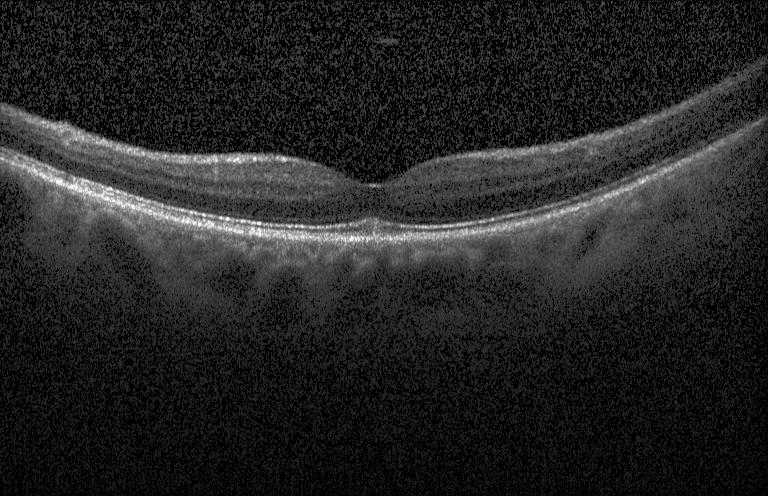

Dx: neither CNV, DME, nor drusen.